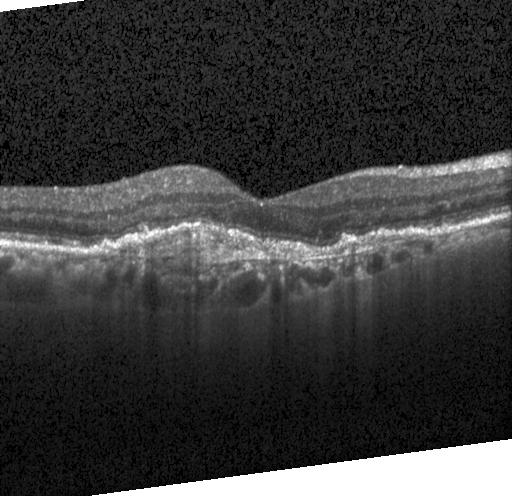

OCT scan showing a choroidal neovascular membrane.